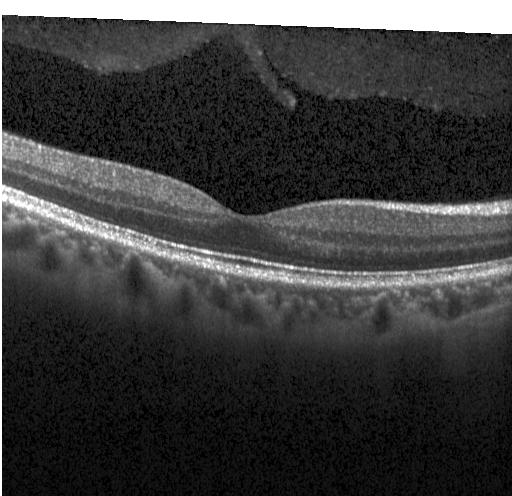
Retinal OCT cross-section showing no choroidal neovascularization, diabetic macular edema, or drusen.